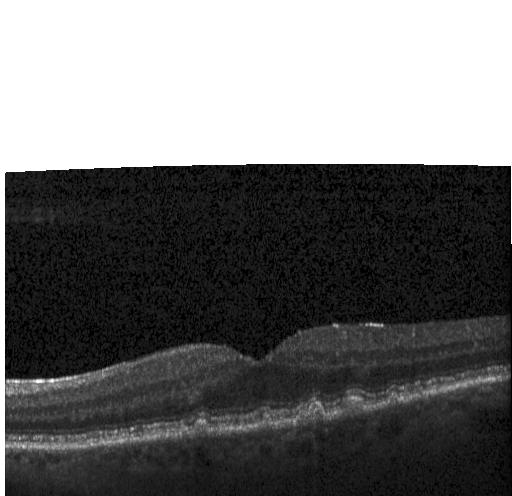

Optical coherence tomography B-scan · fovea-centered — Impression: sub-RPE drusenoid deposits.